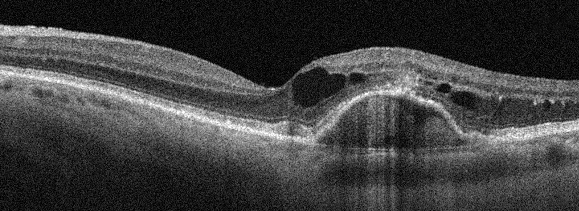
OS · optical coherence tomography B-scan. Dx: age-related macular degeneration.